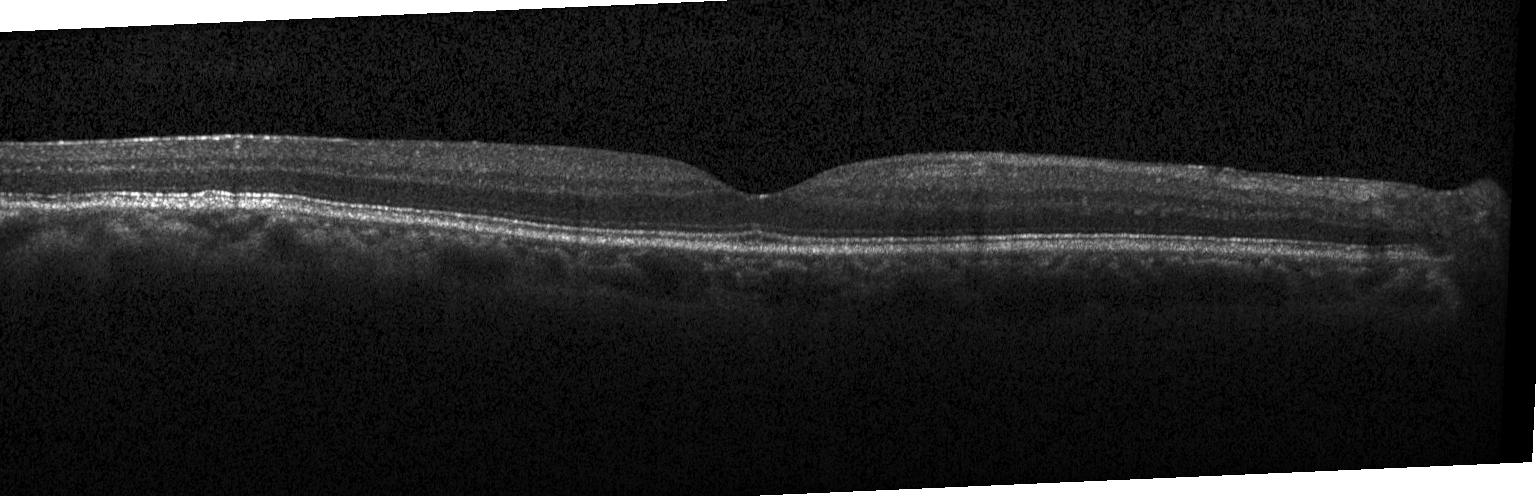

No CNV, DME, or drusen.